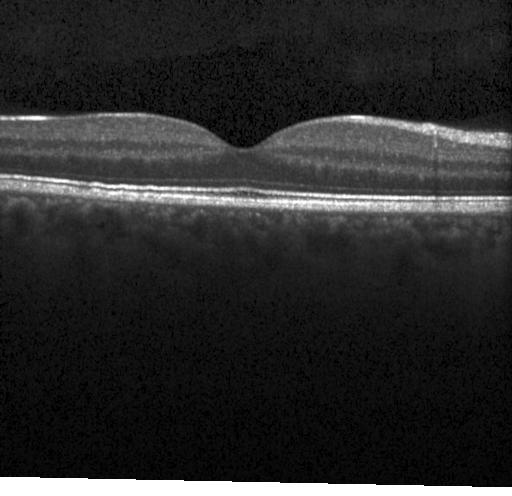

Retinal OCT B-scan.
No CNV, DME, or drusen.